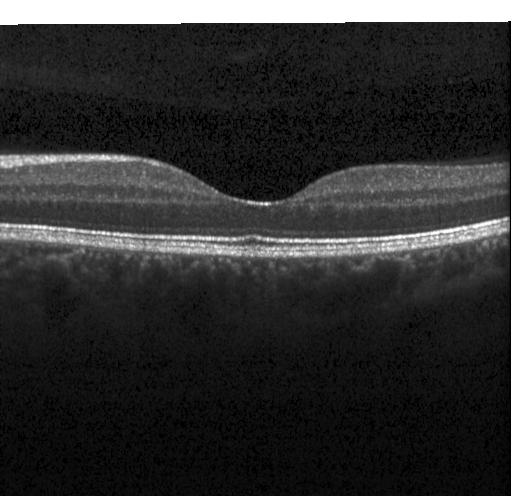
OCT finding: no CNV, no DME, and no drusen.